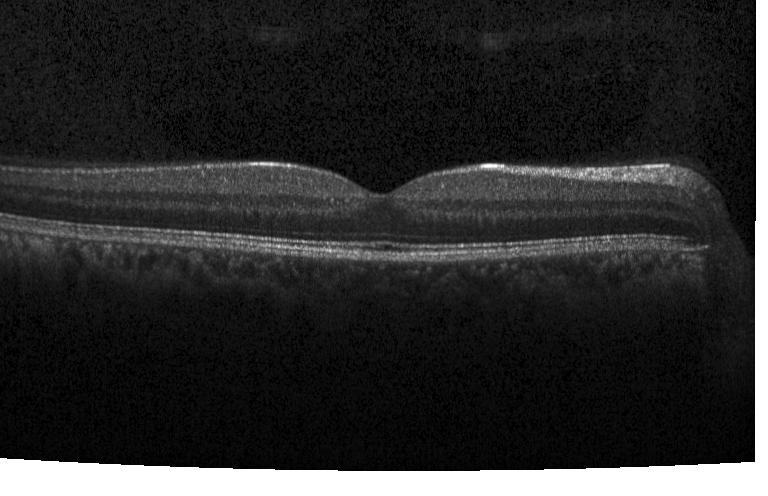
Instrument: Heidelberg Spectralis, OCT line scan, SD-OCT — No choroidal neovascularization, diabetic macular edema, or drusen.